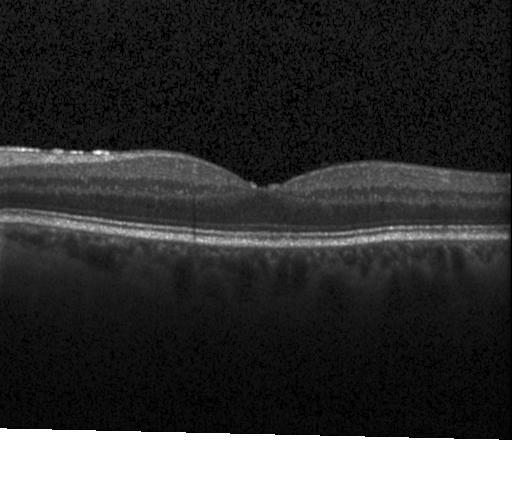 Retinal OCT cross-section. Macular scan.
Finding: no choroidal neovascularization, diabetic macular edema, or drusen.